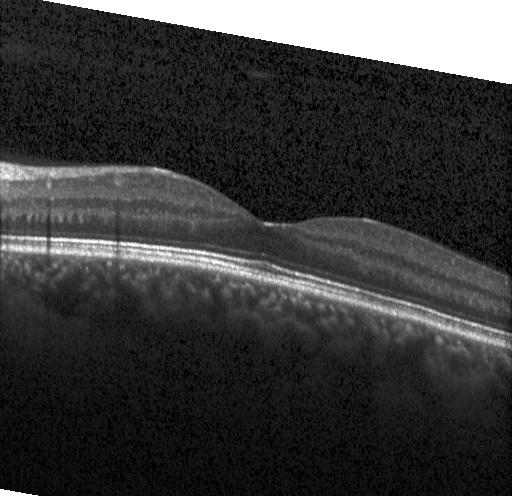
Dx: no choroidal neovascularization, diabetic macular edema, or drusen.